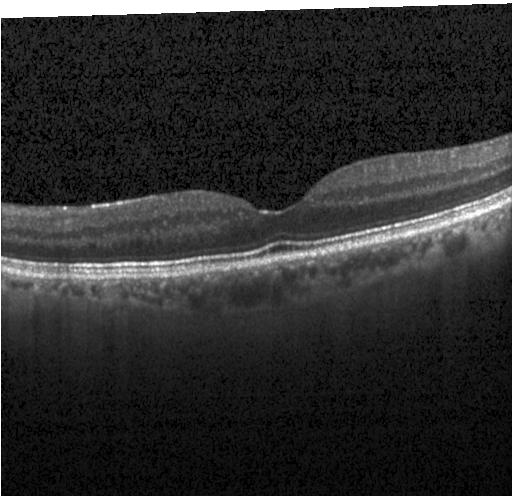
Retinal OCT cross-section showing neither choroidal neovascularization, diabetic macular edema, nor drusen.